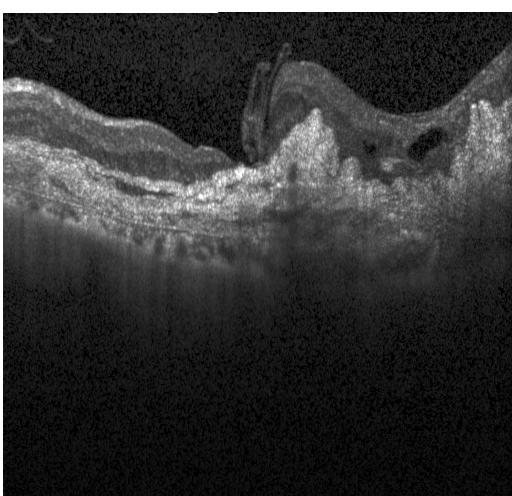
Through the macula; instrument: Heidelberg Spectralis; retinal OCT B-scan; spectral-domain OCT — Finding: choroidal neovascularization.